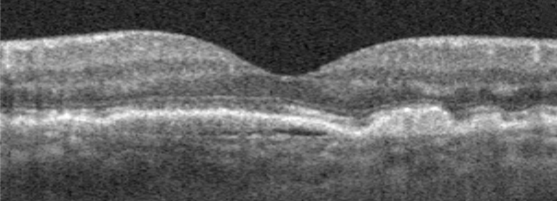 OCT scan showing AMD.